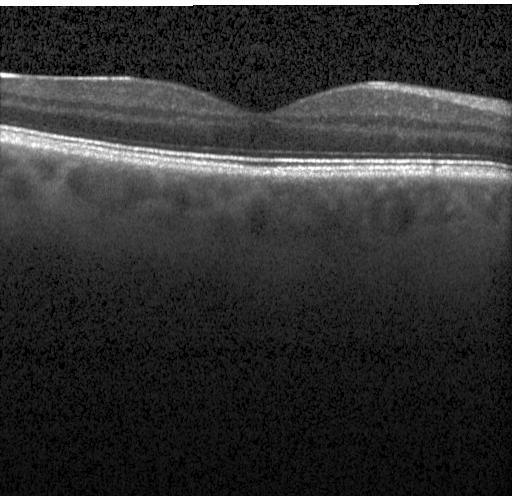
Spectral-domain optical coherence tomography · centered on the fovea · OCT B-scan. Impression: no CNV, DME, or drusen.